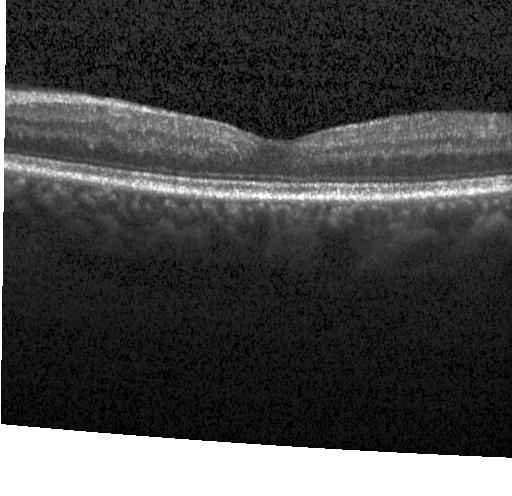

Instrument: Heidelberg Spectralis; optical coherence tomography scan; spectral-domain OCT; fovea-centered — This B-scan demonstrates neither choroidal neovascularization, diabetic macular edema, nor drusen.